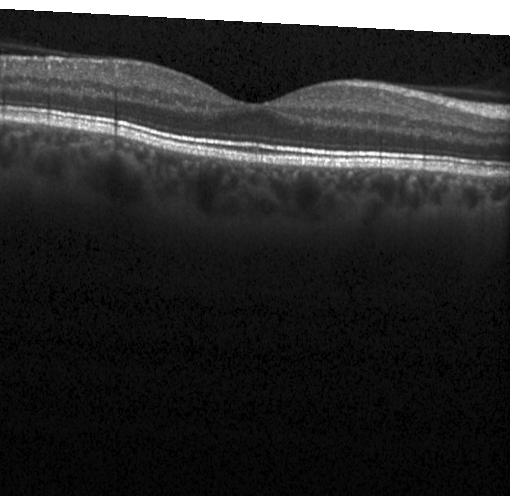 Retinal OCT cross-section · SD-OCT · through the macula.
Impression: neither CNV, DME, nor drusen.